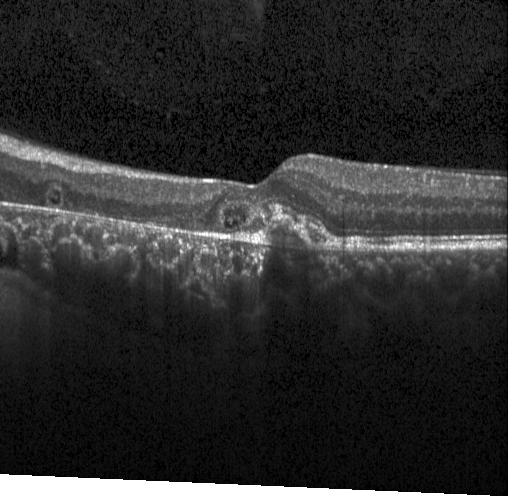 Retinal OCT B-scan, Heidelberg Spectralis OCT system. Diagnosis: a choroidal neovascular membrane.